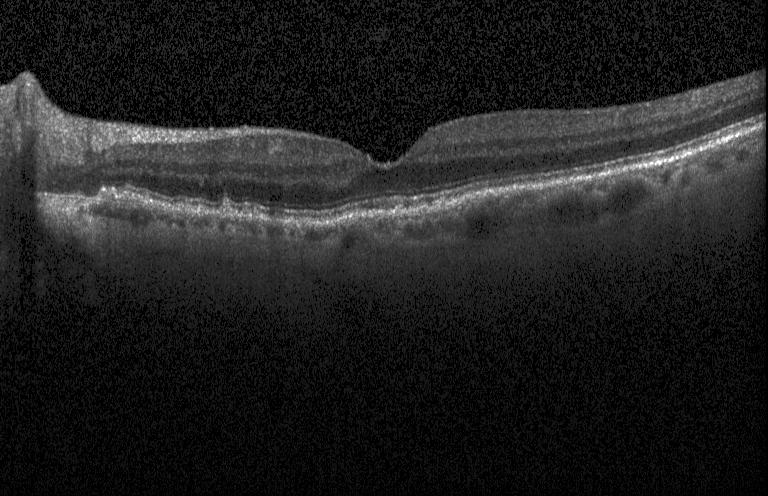 OCT scan showing multiple drusen.